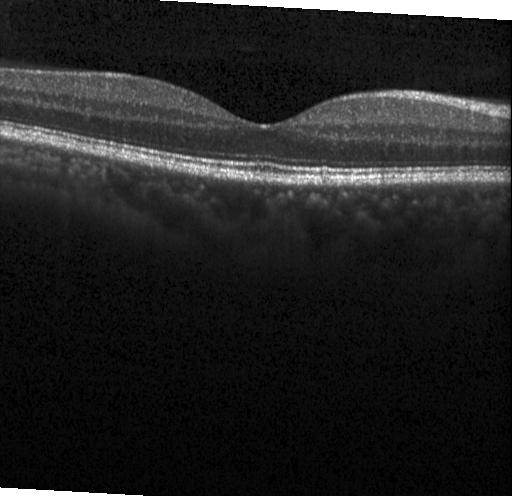 Heidelberg Spectralis OCT system; retinal OCT B-scan. Assessment: no evidence of CNV, DME, or drusen.